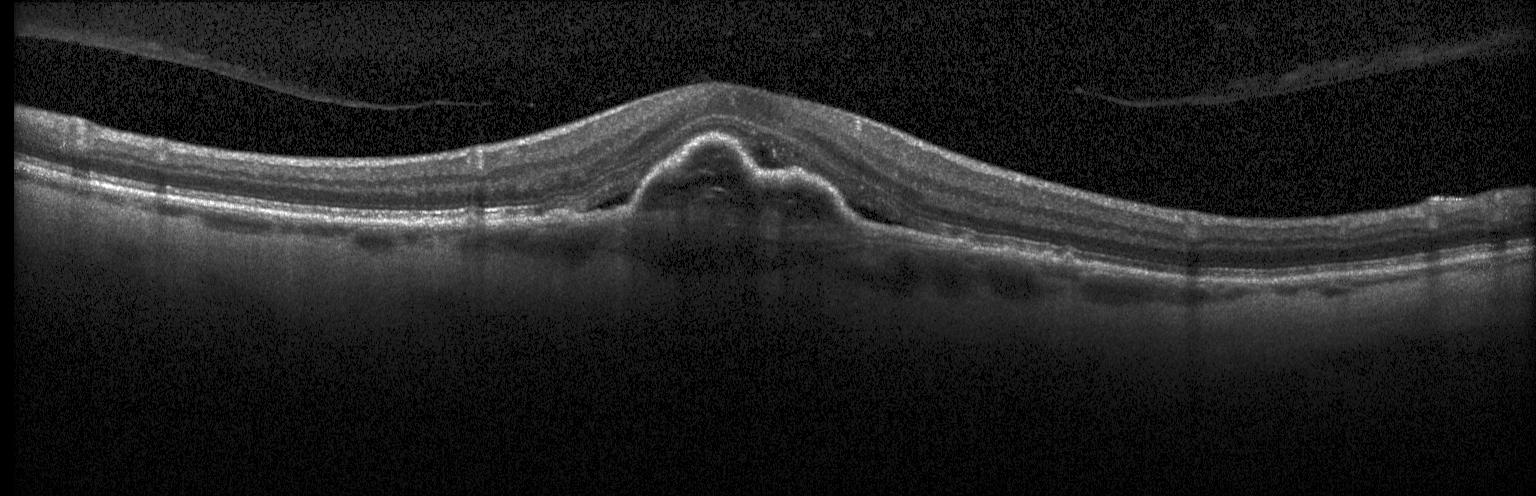

Macular OCT demonstrating a choroidal neovascular membrane.